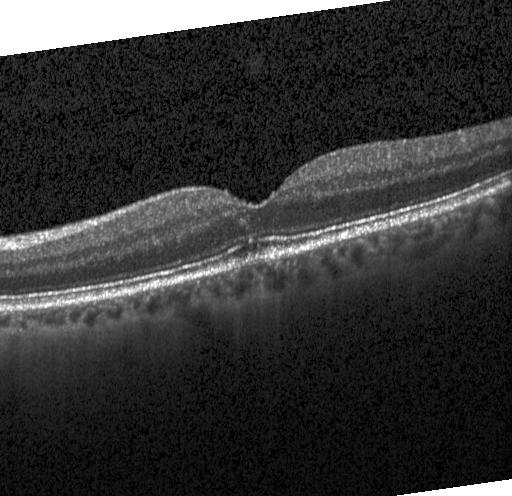
Assessment: CNV.